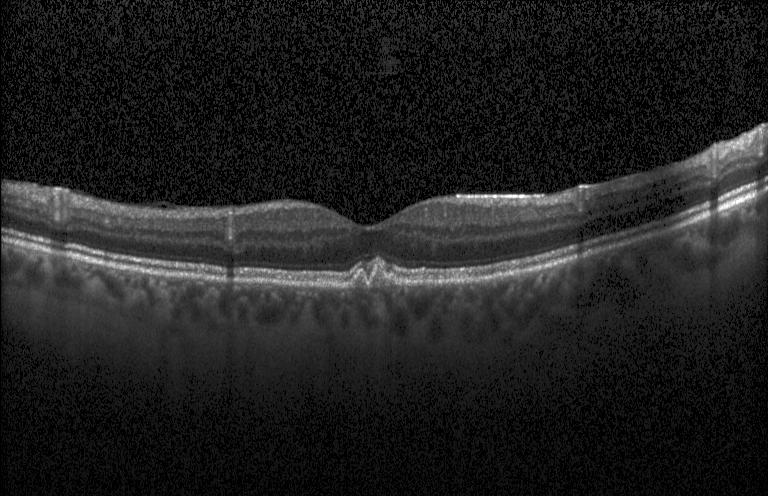 Spectral-domain OCT B-scan: drusen.